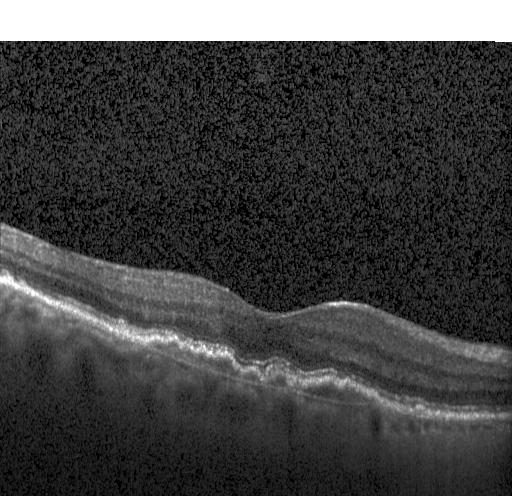 Heidelberg Spectralis · retinal OCT B-scan · horizontal scan through the fovea · spectral-domain OCT — Impression: a choroidal neovascular membrane.